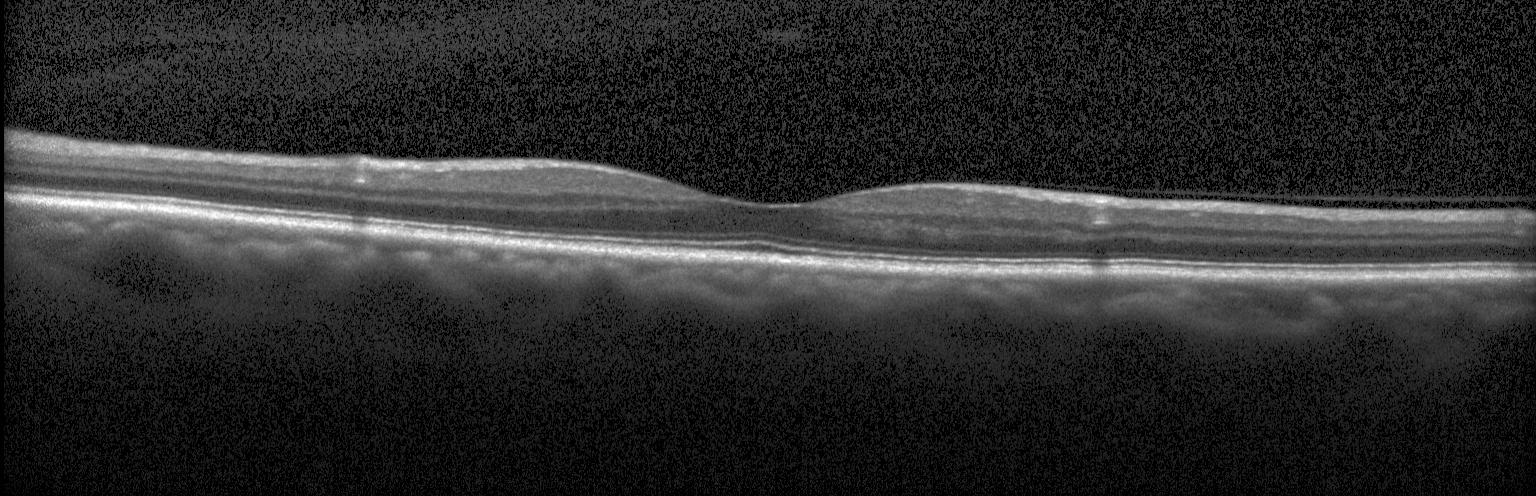 Finding: no choroidal neovascularization, diabetic macular edema, or drusen.